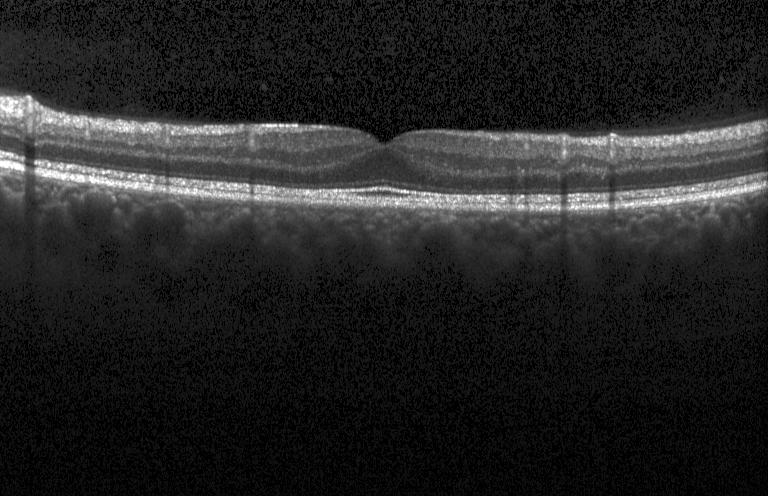

Fovea-centered; spectral-domain optical coherence tomography; Heidelberg Spectralis; optical coherence tomography scan.
Macular OCT: no choroidal neovascularization, no diabetic macular edema, and no drusen.